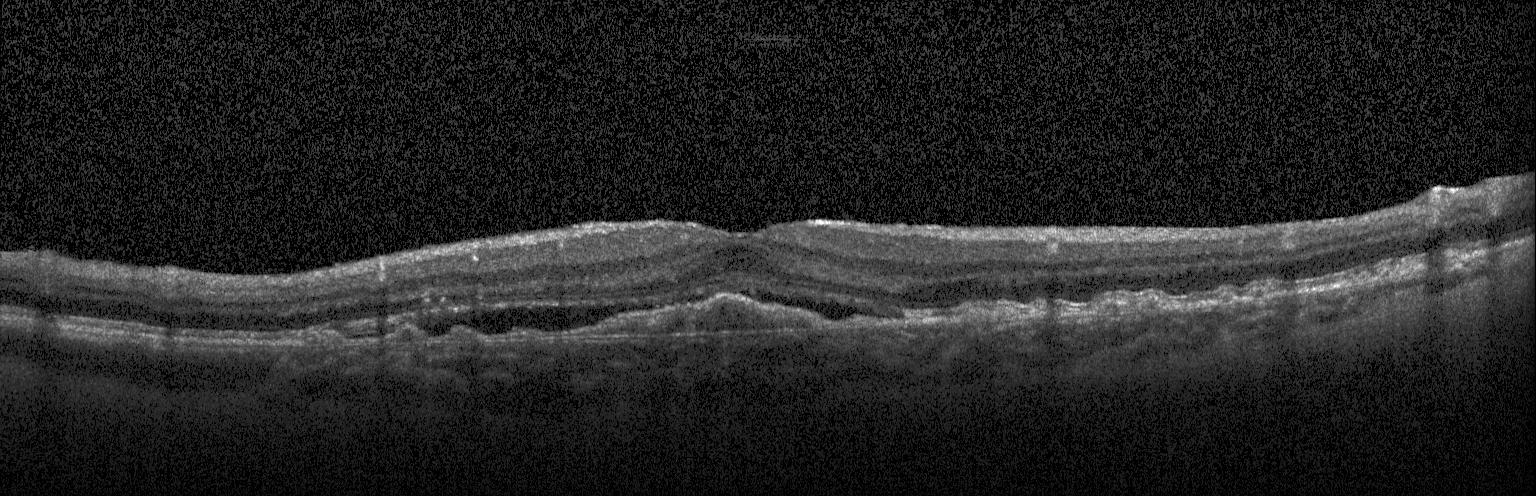
Finding: choroidal neovascularization.